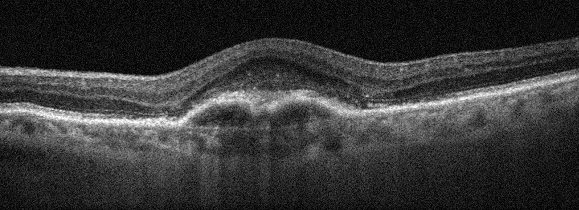

Optical coherence tomography scan, OS. Assessment: age-related macular degeneration.